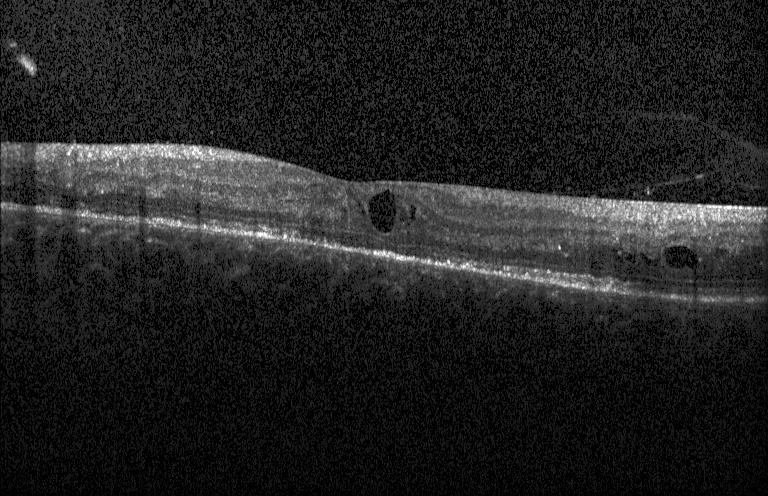 Macular scan; OCT line scan; spectral-domain optical coherence tomography; acquired on a Heidelberg Spectralis.
Finding: DME.